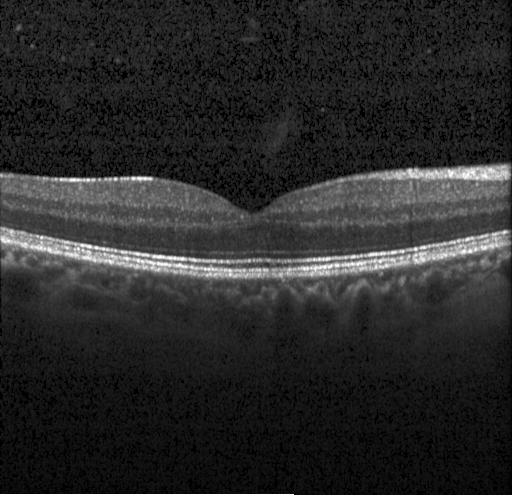

Acquired on a Heidelberg Spectralis. Centered on the fovea. Optical coherence tomography scan. Spectral-domain OCT.
Assessment: no choroidal neovascularization, no diabetic macular edema, and no drusen.